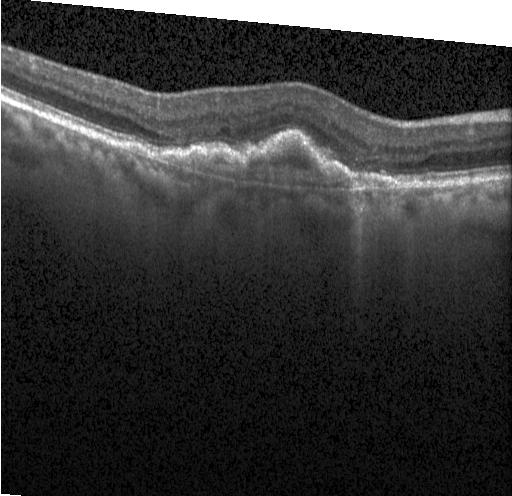
OCT line scan, Heidelberg Spectralis OCT system.
Diagnosis: a choroidal neovascular membrane.